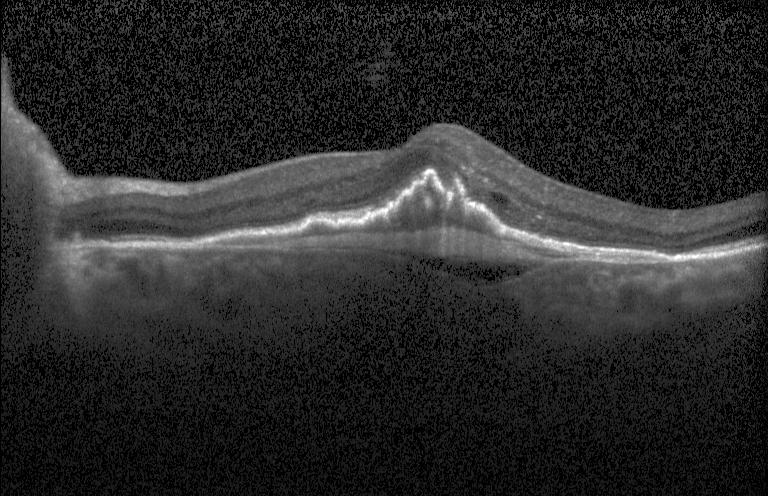 SD-OCT. OCT B-scan.
This B-scan demonstrates choroidal neovascularization (CNV).